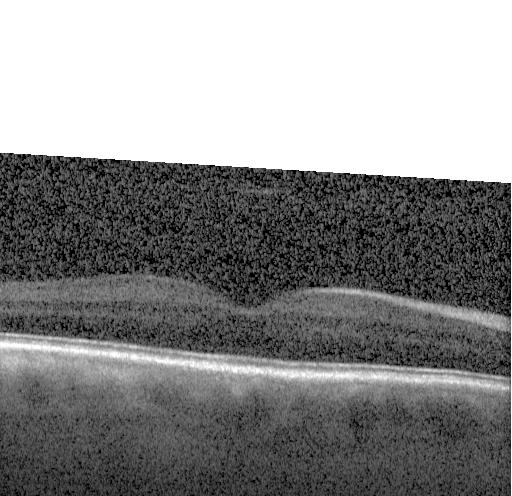

Heidelberg Spectralis OCT system. OCT line scan. Assessment: no CNV, no DME, and no drusen.